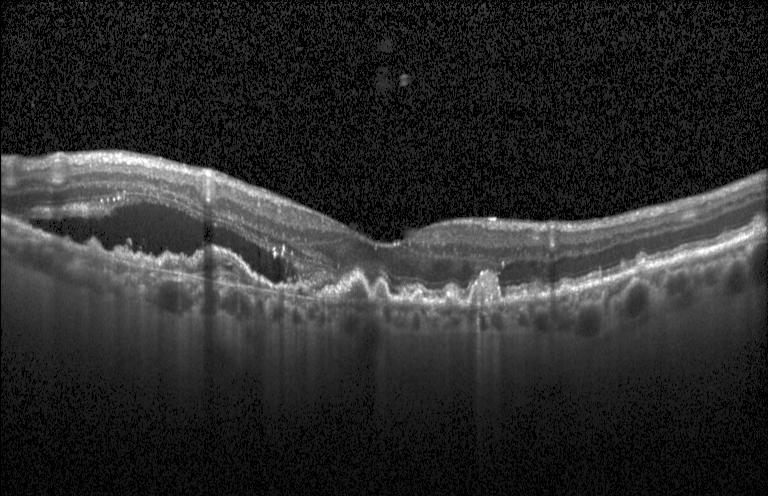 The scan shows CNV.